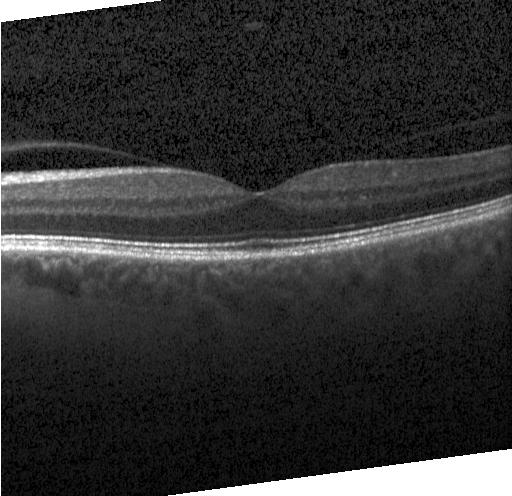
SD-OCT; fovea-centered; OCT line scan. Finding: no CNV, DME, or drusen.